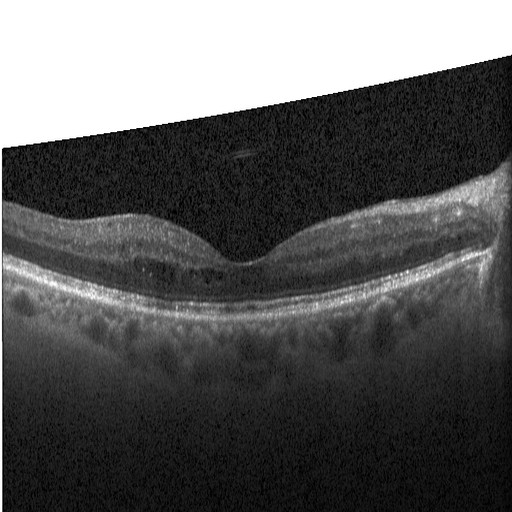 Spectral-domain optical coherence tomography; retinal OCT cross-section; instrument: Heidelberg Spectralis; fovea-centered — Finding: DME.